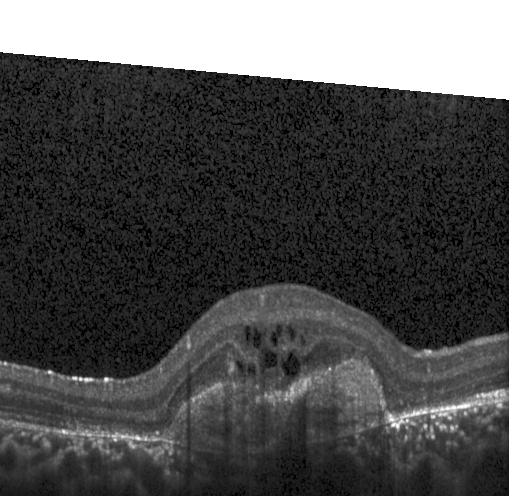 Fovea-centered. OCT B-scan. Heidelberg Spectralis — Finding: a choroidal neovascular membrane.